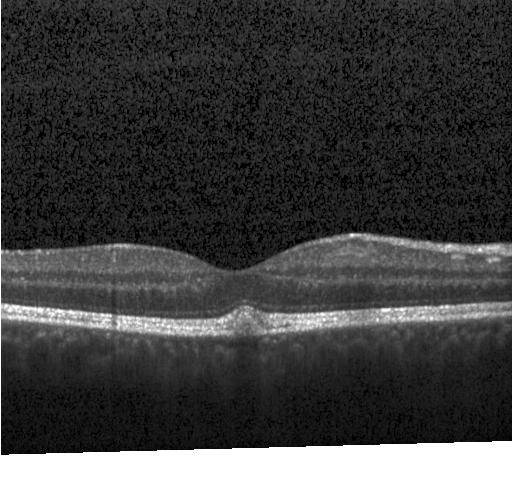
Finding: multiple drusen.